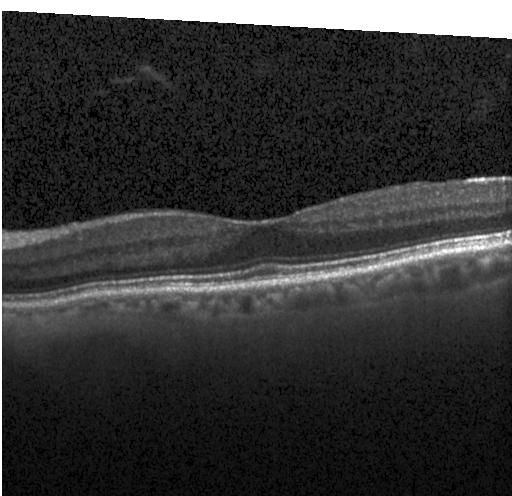
Retinal OCT cross-section; horizontal scan through the fovea. This B-scan demonstrates no choroidal neovascularization, no diabetic macular edema, and no drusen.